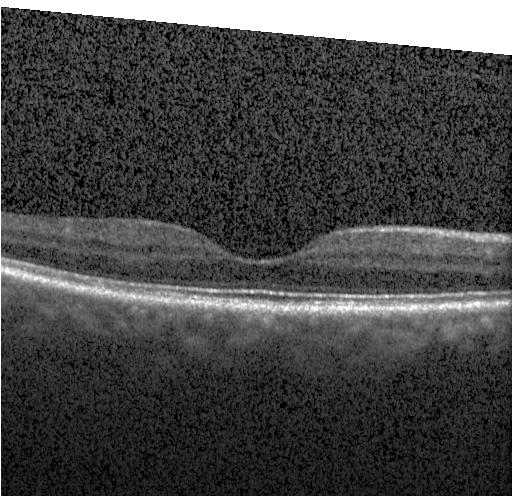
OCT finding: no evidence of choroidal neovascularization, diabetic macular edema, or drusen.